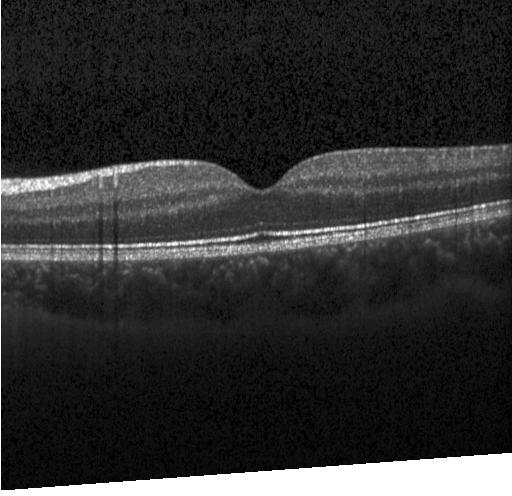

SD-OCT. Retinal OCT cross-section. Diagnosis: no evidence of CNV, DME, or drusen.